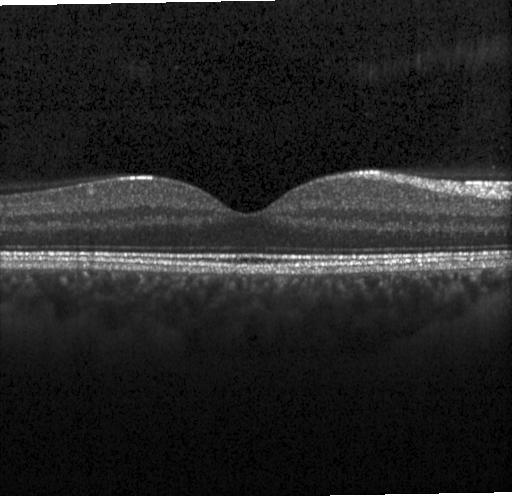
Optical coherence tomography scan. Assessment: neither choroidal neovascularization, diabetic macular edema, nor drusen.